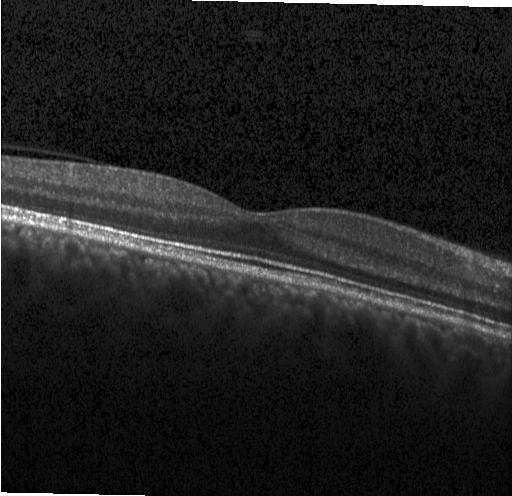
Diagnosis: no evidence of choroidal neovascularization, diabetic macular edema, or drusen.